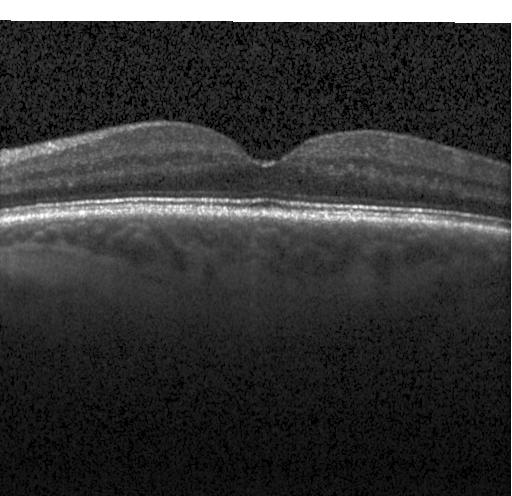
SD-OCT · horizontal scan through the fovea · OCT B-scan · Heidelberg Spectralis.
This B-scan demonstrates no CNV, no DME, and no drusen.